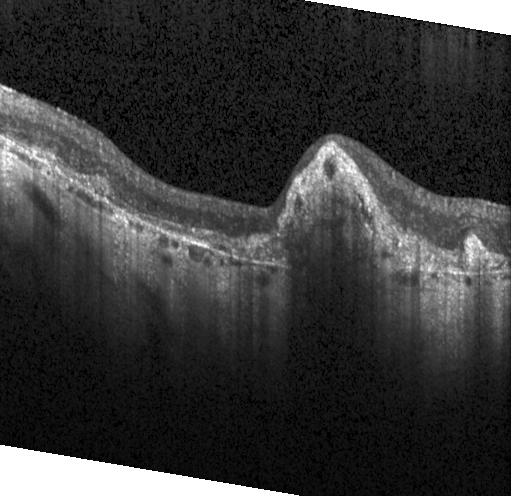

Heidelberg Spectralis OCT system, spectral-domain optical coherence tomography, retinal OCT B-scan, fovea-centered — Finding: a choroidal neovascular membrane.